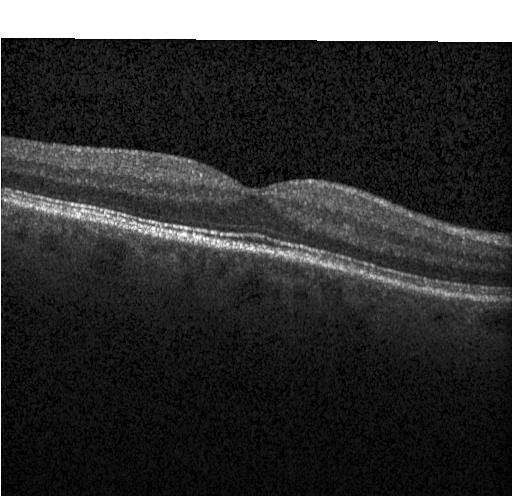 Retinal OCT B-scan, Heidelberg Spectralis OCT system
Diagnosis: no CNV, DME, or drusen.